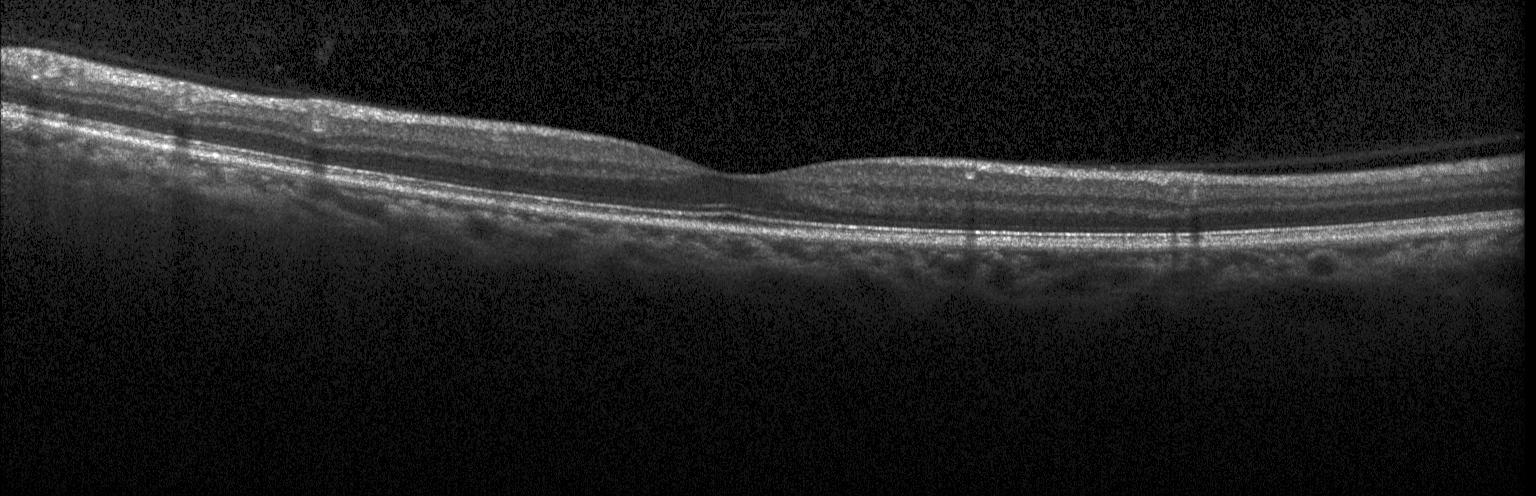

Centered on the fovea, optical coherence tomography B-scan. OCT finding: no CNV, DME, or drusen.